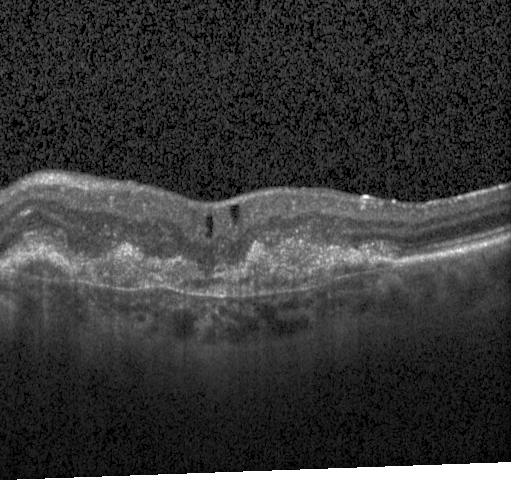
Spectral-domain optical coherence tomography · optical coherence tomography B-scan · acquired on a Heidelberg Spectralis · centered on the fovea. Diagnosis: CNV.